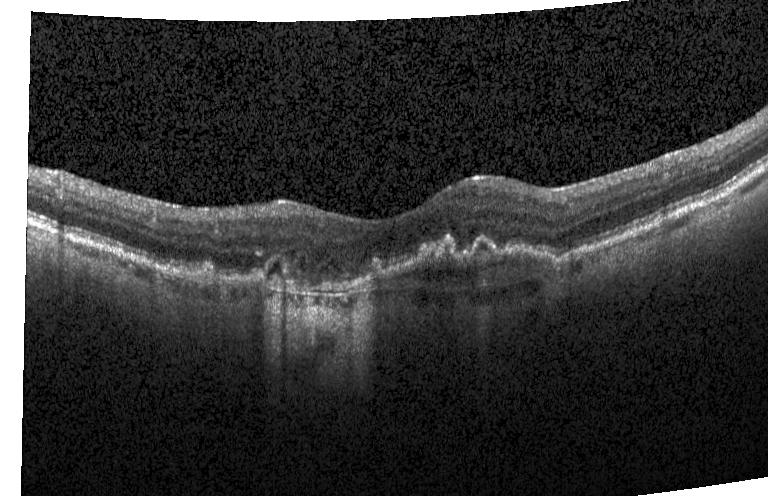
OCT line scan · through the macula — This B-scan demonstrates CNV.